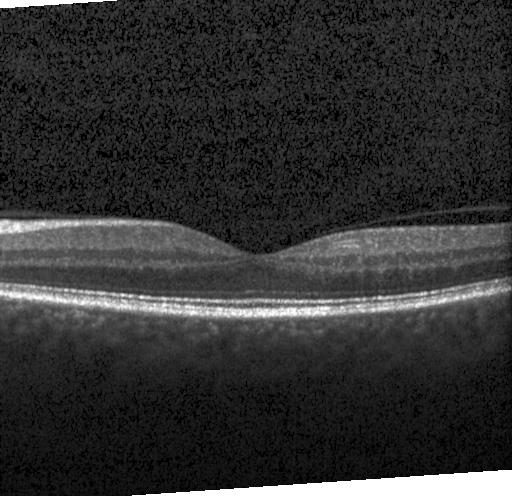 OCT B-scan
Impression: no CNV, DME, or drusen.